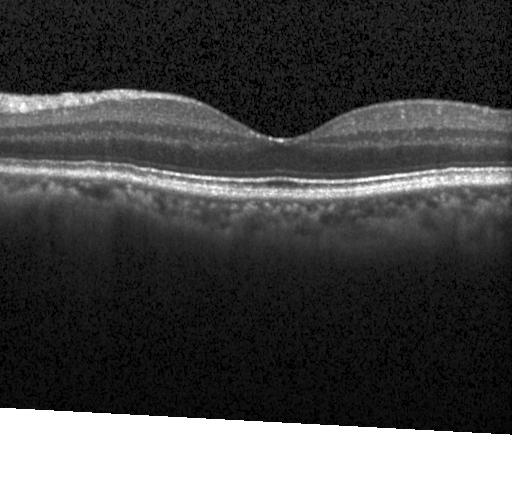 Macular scan, OCT line scan, SD-OCT
Impression: no choroidal neovascularization, no diabetic macular edema, and no drusen.